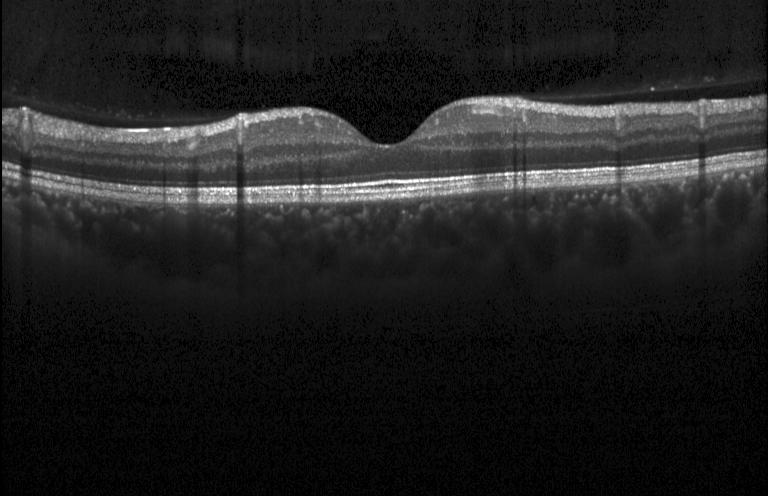

Retinal OCT cross-section showing no choroidal neovascularization, diabetic macular edema, or drusen.